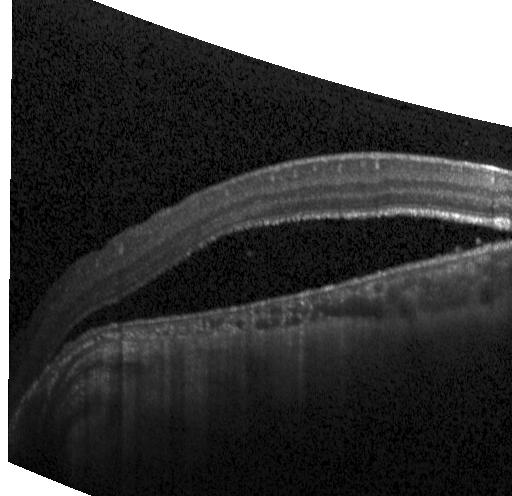
Finding: choroidal neovascularization.